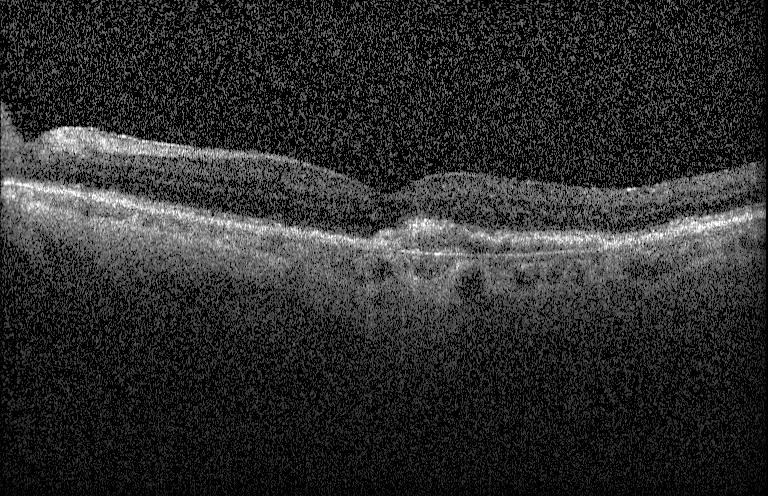

Finding: a choroidal neovascular membrane.